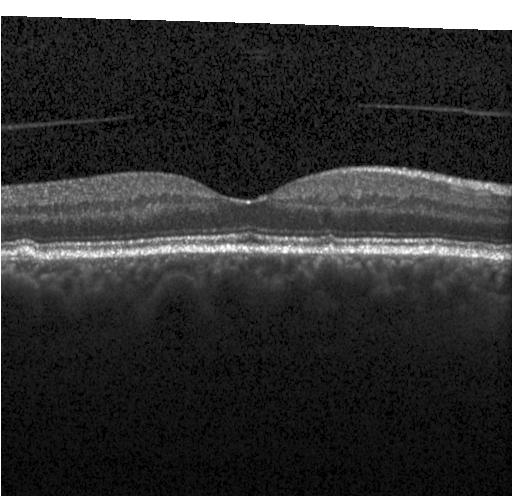 The scan shows multiple drusen.